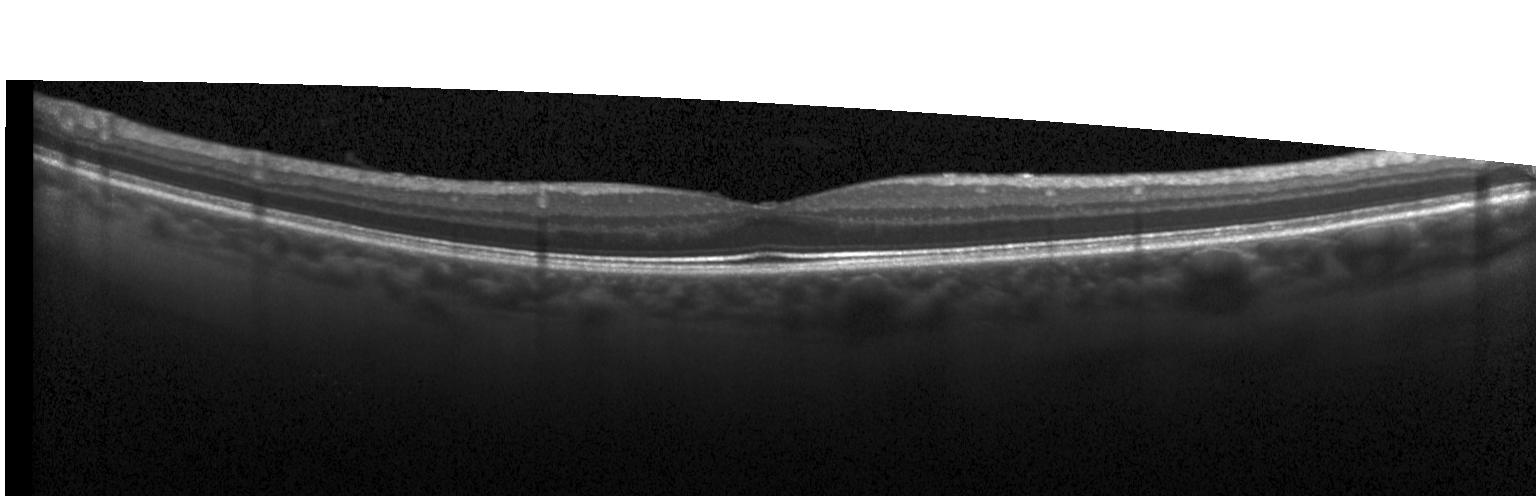

OCT B-scan.
OCT finding: neither CNV, DME, nor drusen.